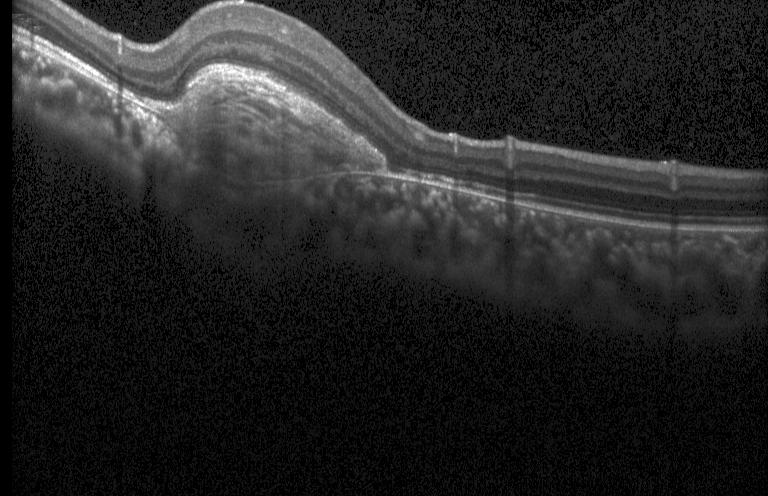 OCT finding: a choroidal neovascular membrane.